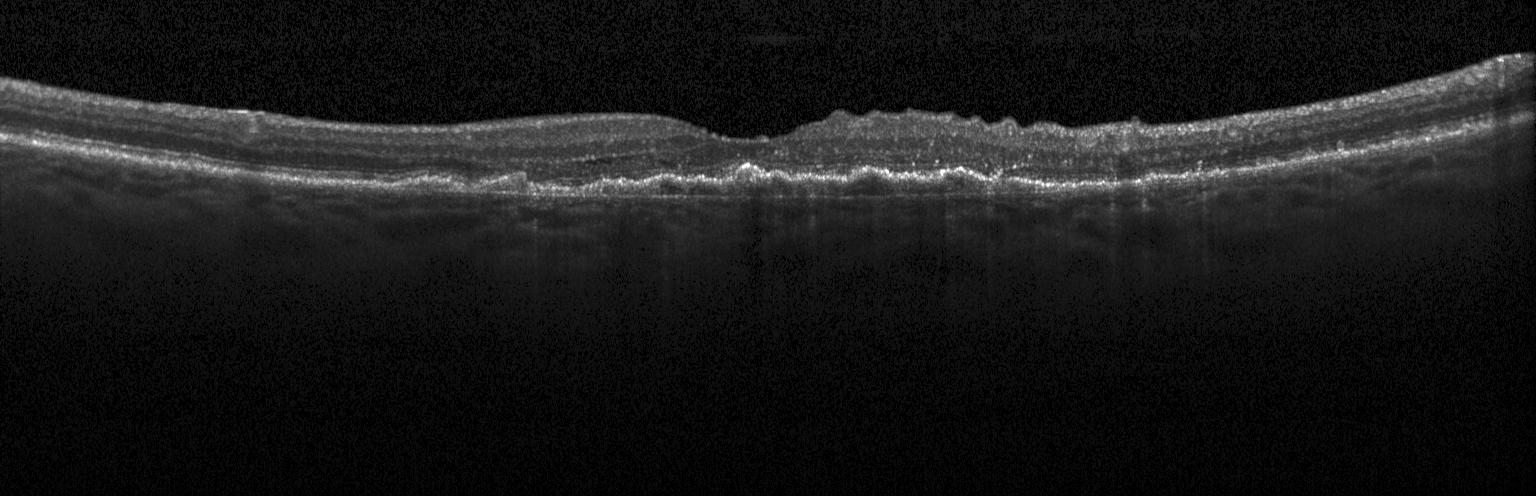 Spectral-domain optical coherence tomography; centered on the fovea; OCT line scan; Heidelberg Spectralis OCT system. Finding: choroidal neovascularization (CNV).